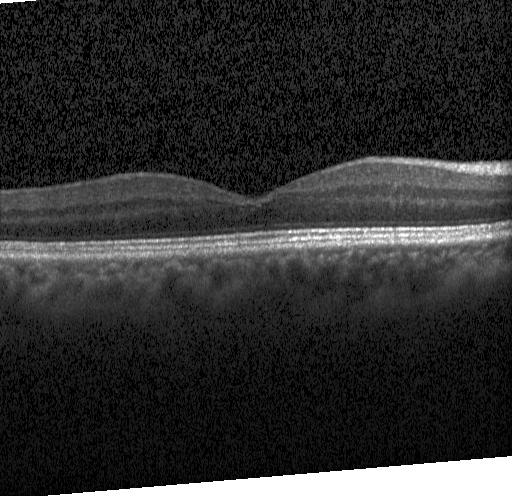
Macular OCT demonstrating neither choroidal neovascularization, diabetic macular edema, nor drusen.